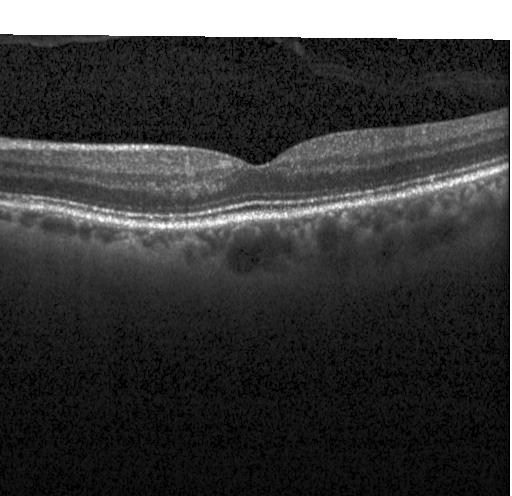 Retinal OCT cross-section, SD-OCT, horizontal scan through the fovea — Finding: no choroidal neovascularization, diabetic macular edema, or drusen.